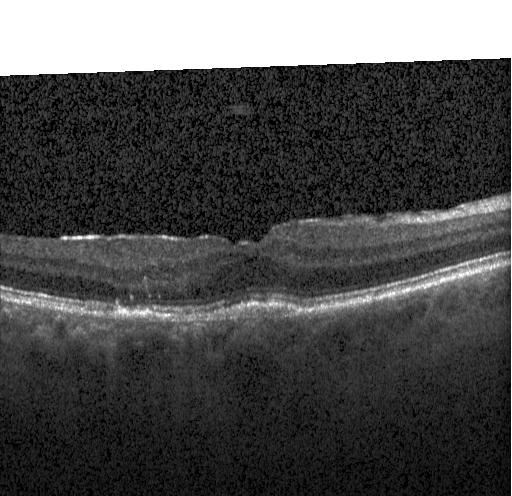

Heidelberg Spectralis. Retinal OCT cross-section.
Impression: a choroidal neovascular membrane.